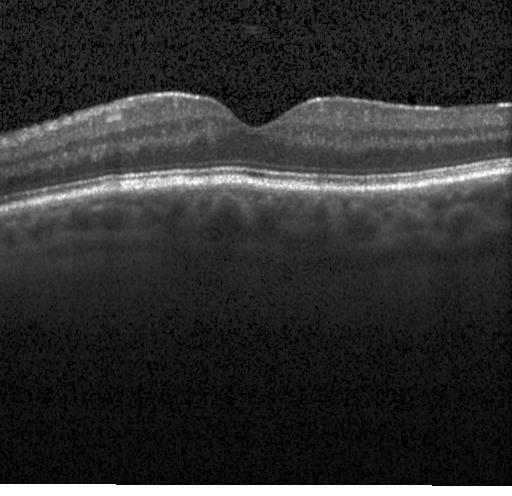

Optical coherence tomography scan
Macular OCT: no choroidal neovascularization, no diabetic macular edema, and no drusen.